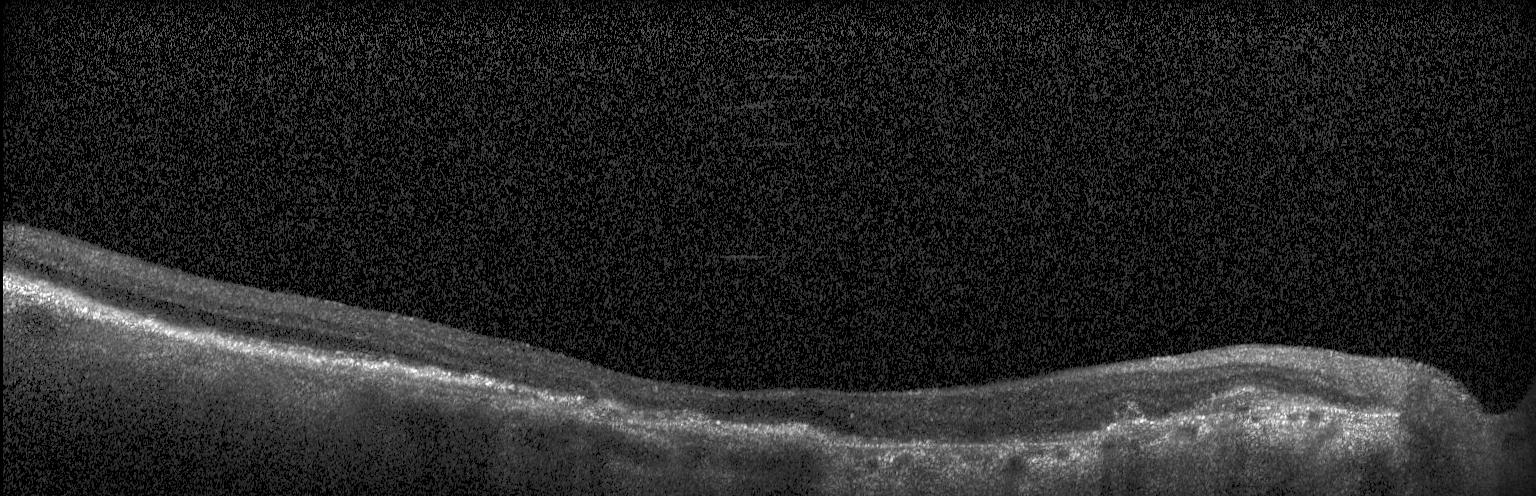
SD-OCT · Heidelberg Spectralis · optical coherence tomography B-scan — Choroidal neovascularization (CNV).